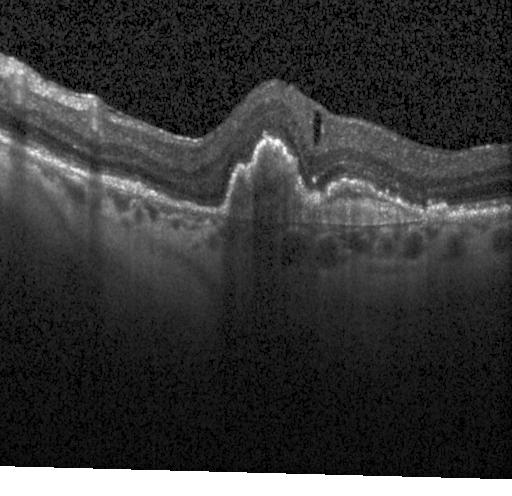 SD-OCT. Retinal OCT cross-section.
OCT finding: a choroidal neovascular membrane.